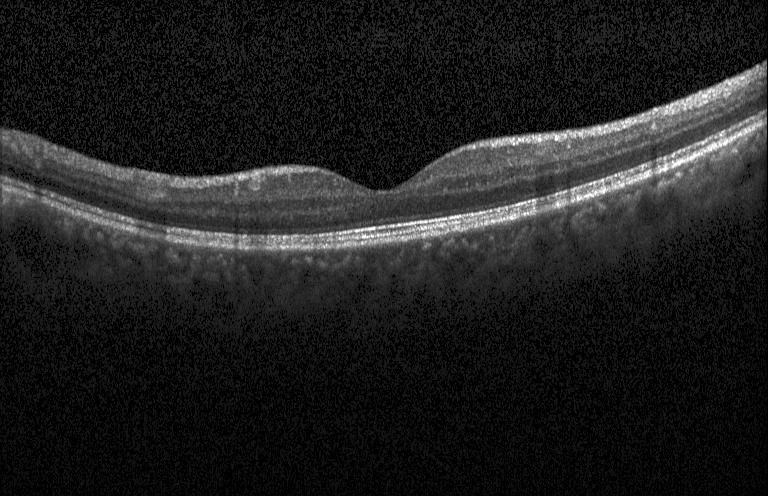

Retinal OCT cross-section, spectral-domain OCT
This B-scan demonstrates neither choroidal neovascularization, diabetic macular edema, nor drusen.